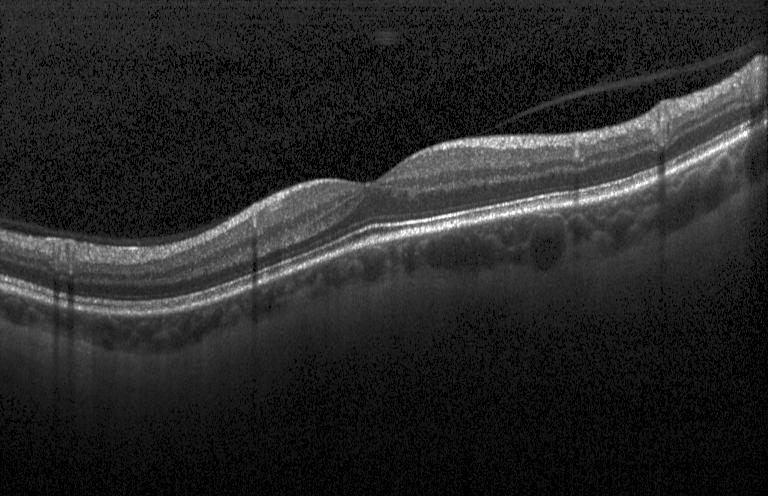 OCT B-scan showing neither choroidal neovascularization, diabetic macular edema, nor drusen.